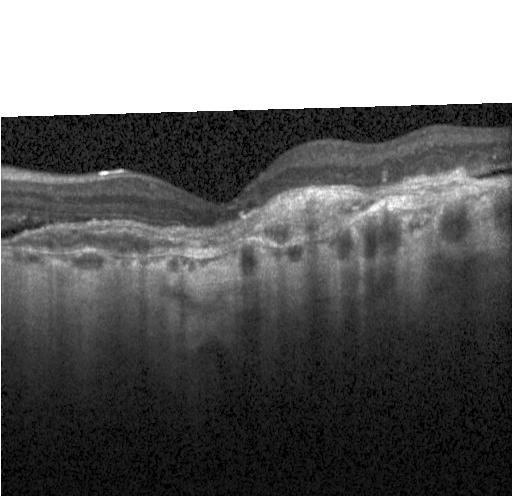

OCT line scan.
Finding: a choroidal neovascular membrane.